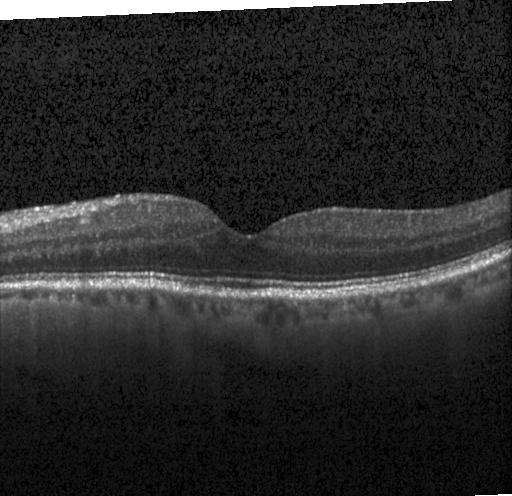

Spectral-domain optical coherence tomography · OCT line scan.
Dx: neither choroidal neovascularization, diabetic macular edema, nor drusen.